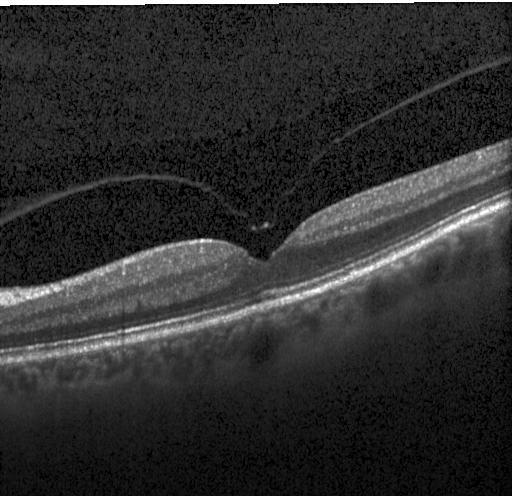

SD-OCT, optical coherence tomography scan, fovea-centered.
Assessment: no CNV, DME, or drusen.